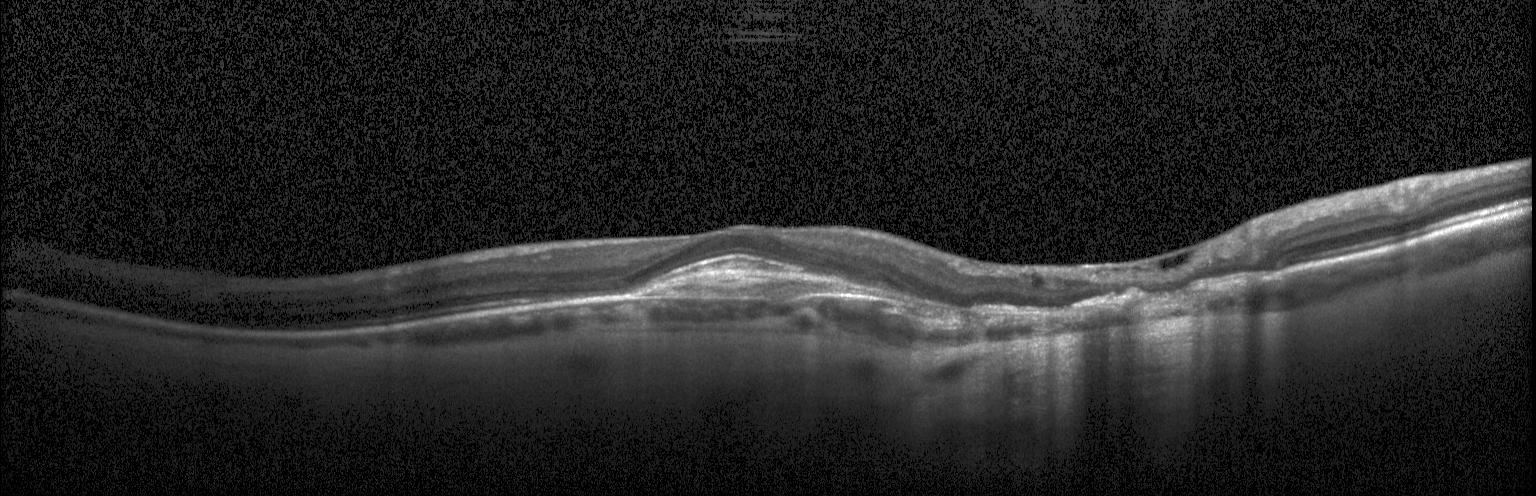

SD-OCT, fovea-centered, optical coherence tomography scan.
Impression: a choroidal neovascular membrane.